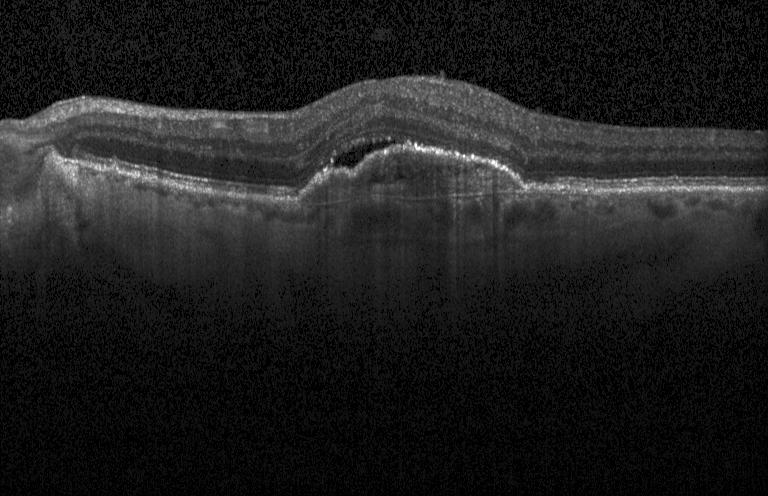

SD-OCT. Fovea-centered. Retinal OCT cross-section. Heidelberg Spectralis. This B-scan demonstrates a choroidal neovascular membrane.